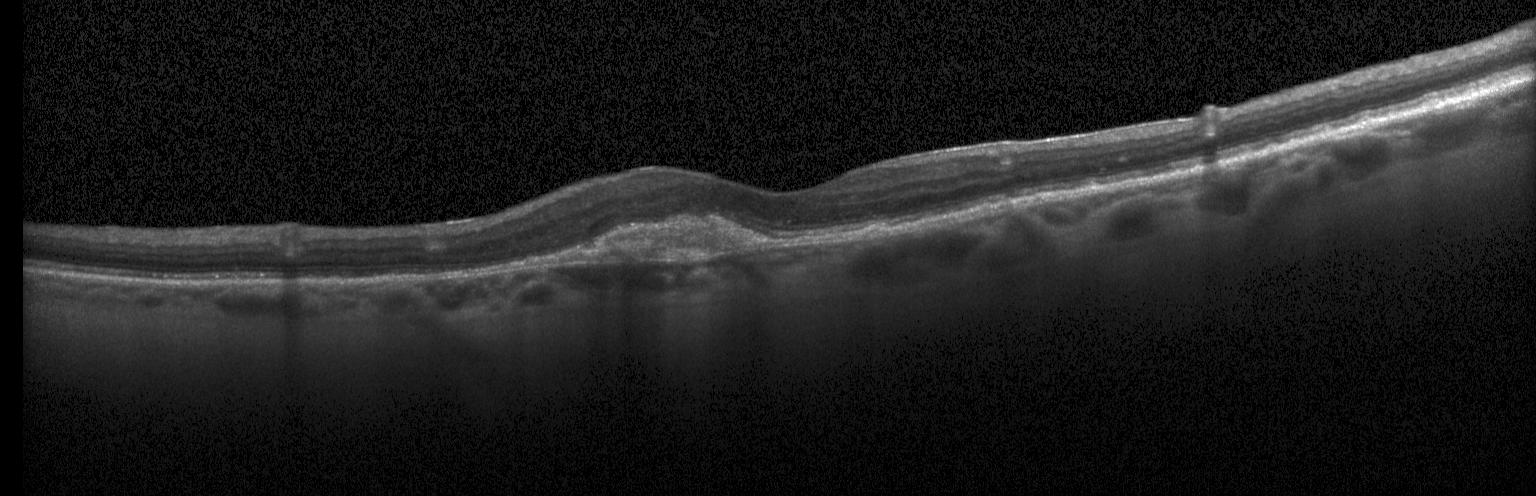

SD-OCT · optical coherence tomography scan · fovea-centered. Finding: a choroidal neovascular membrane.